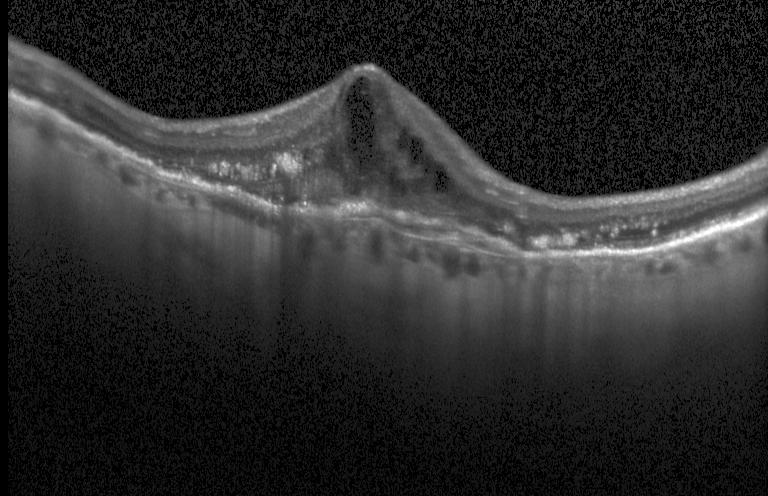

Optical coherence tomography B-scan, macular scan
Impression: a choroidal neovascular membrane.